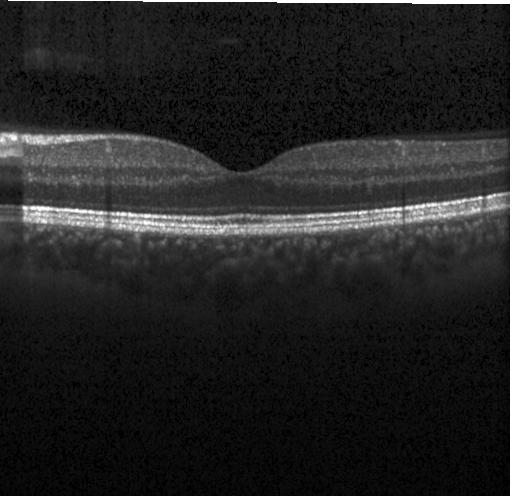
This B-scan demonstrates no choroidal neovascularization, no diabetic macular edema, and no drusen.